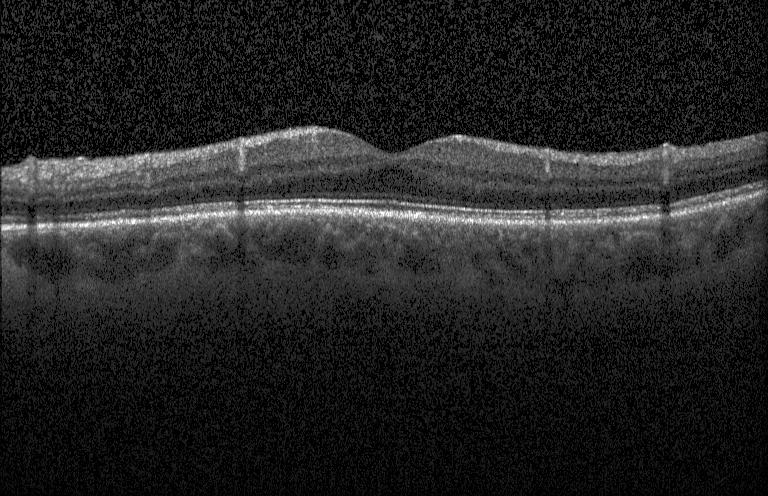
Heidelberg Spectralis OCT system, centered on the fovea, SD-OCT, OCT B-scan. Assessment: neither choroidal neovascularization, diabetic macular edema, nor drusen.